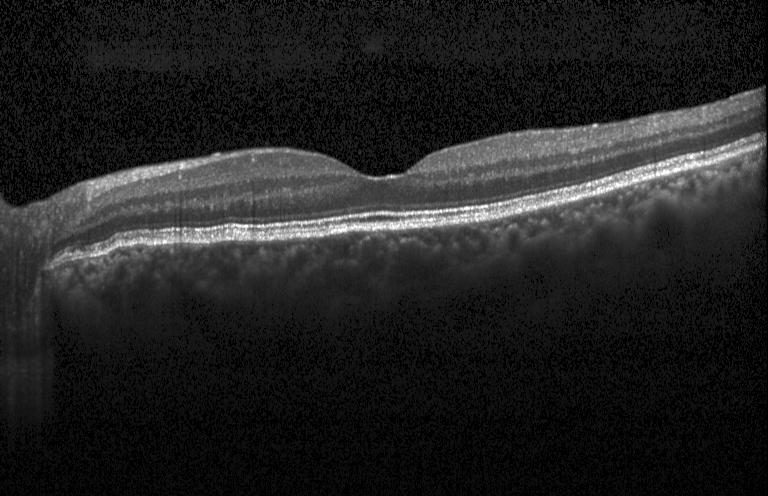 OCT B-scan · spectral-domain optical coherence tomography · Heidelberg Spectralis · fovea-centered — Finding: no evidence of CNV, DME, or drusen.